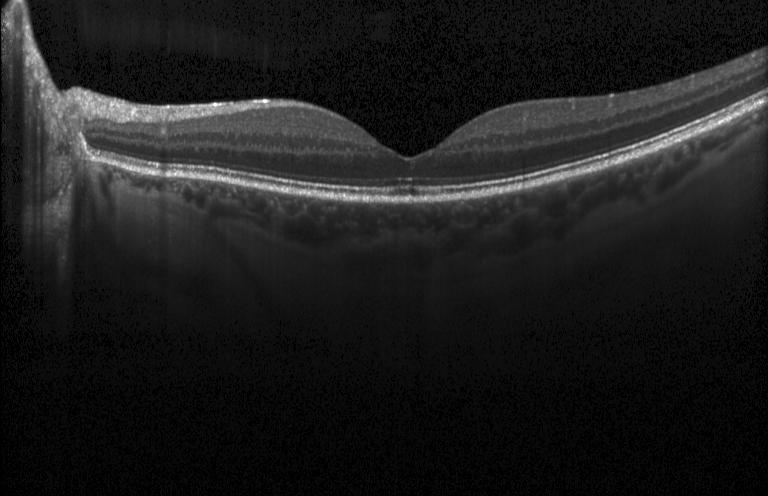
Spectral-domain OCT. Optical coherence tomography B-scan. Heidelberg Spectralis. Centered on the fovea. Assessment: no choroidal neovascularization, no diabetic macular edema, and no drusen.